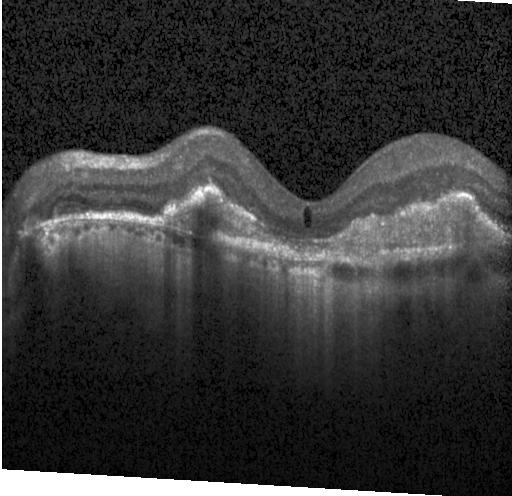
Retinal OCT cross-section showing choroidal neovascularization.